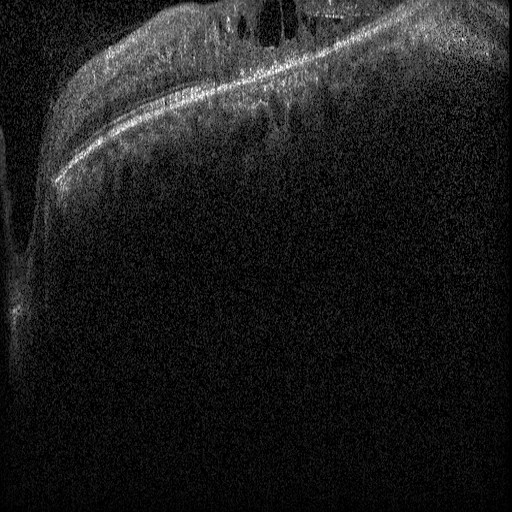
OCT B-scan, fovea-centered
The scan shows DME.